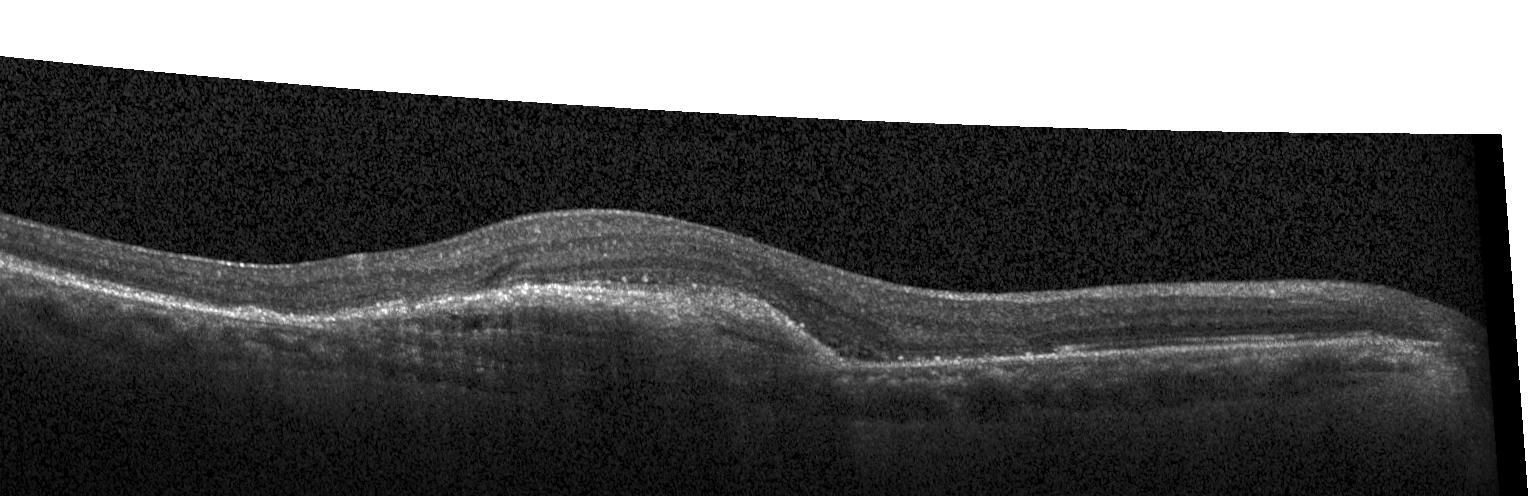

OCT B-scan showing choroidal neovascularization.